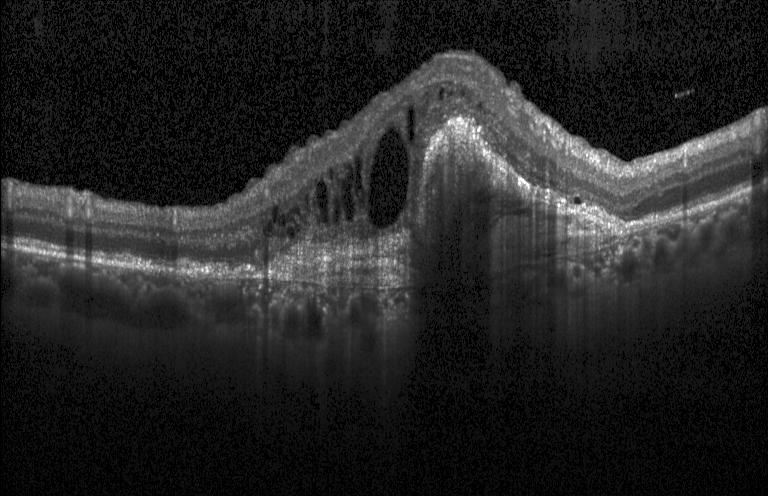

Heidelberg Spectralis · retinal OCT B-scan · through the macula
Finding: a choroidal neovascular membrane.